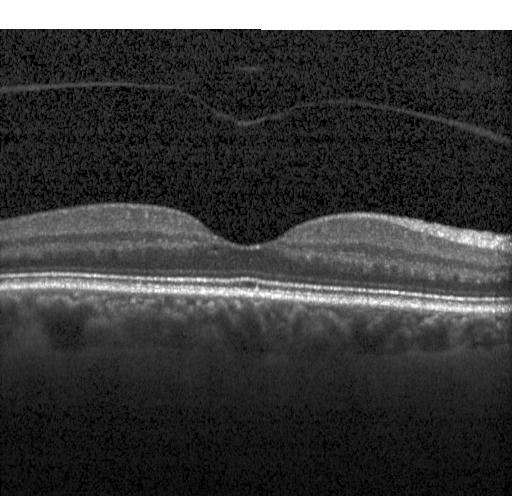

OCT line scan · instrument: Heidelberg Spectralis. Macular OCT: no choroidal neovascularization, diabetic macular edema, or drusen.